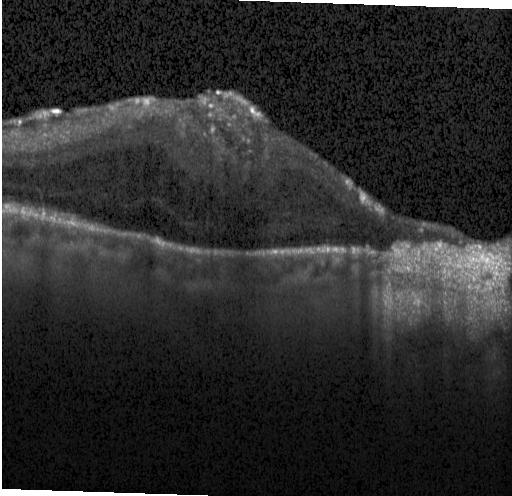

OCT B-scan; fovea-centered. The scan shows DME.